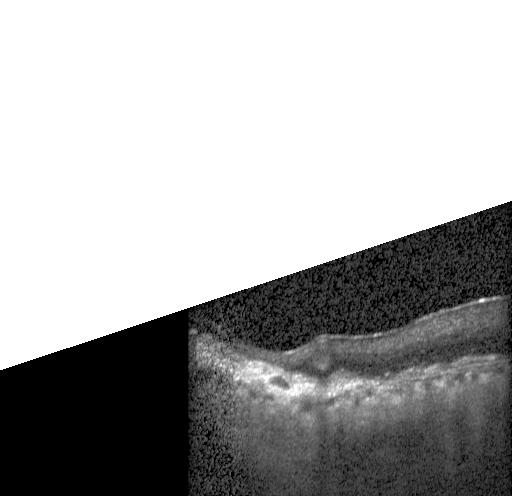 Dx: a choroidal neovascular membrane.